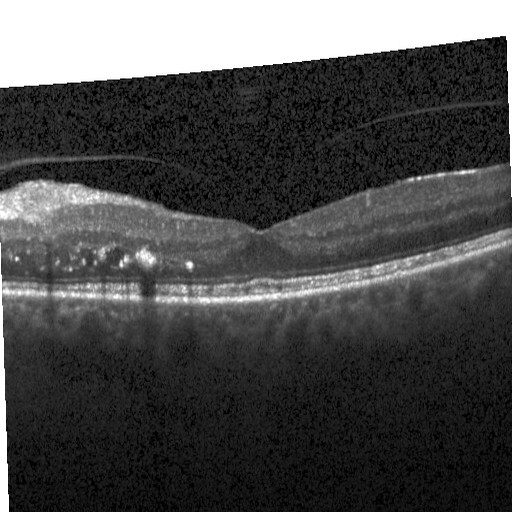 Dx: diabetic macular edema (DME).